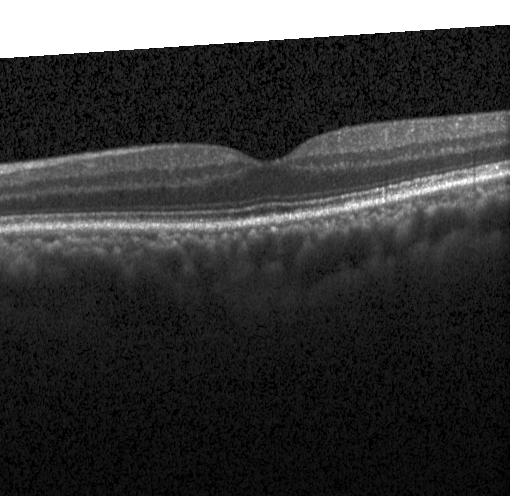

Optical coherence tomography scan · acquired on a Heidelberg Spectralis
Impression: no choroidal neovascularization, no diabetic macular edema, and no drusen.